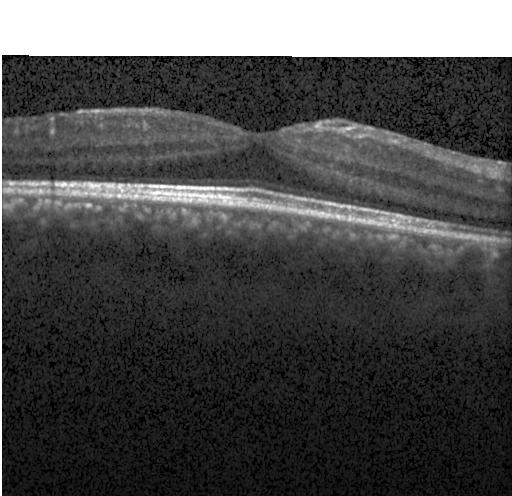 Assessment: neither CNV, DME, nor drusen.